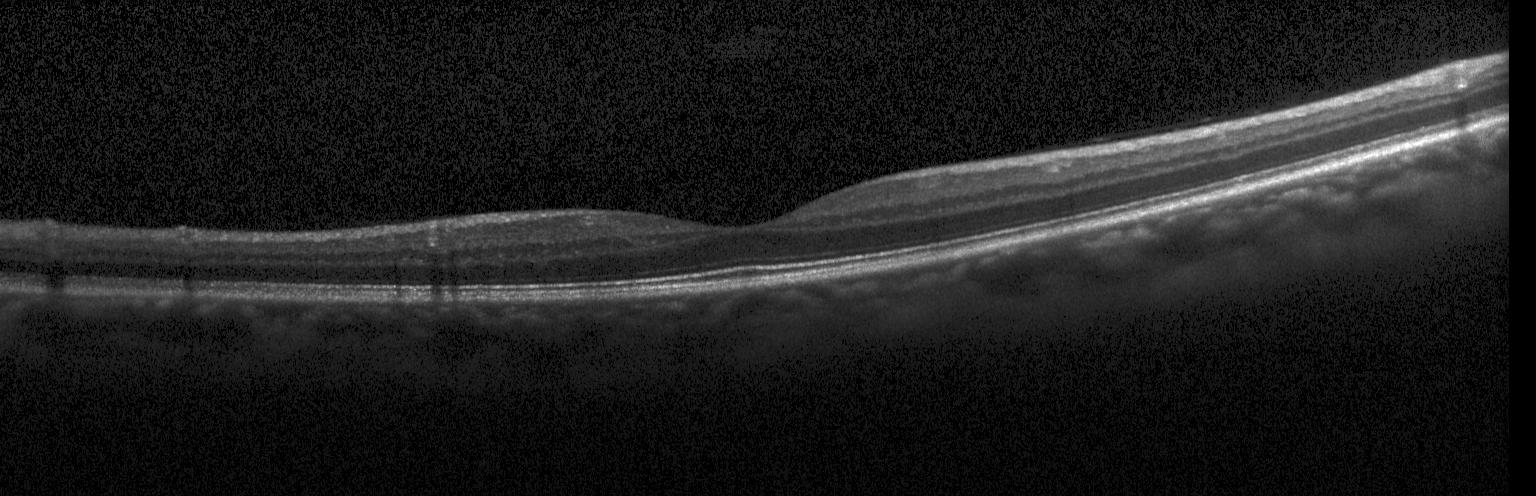
Spectral-domain OCT · optical coherence tomography B-scan. Finding: no choroidal neovascularization, no diabetic macular edema, and no drusen.